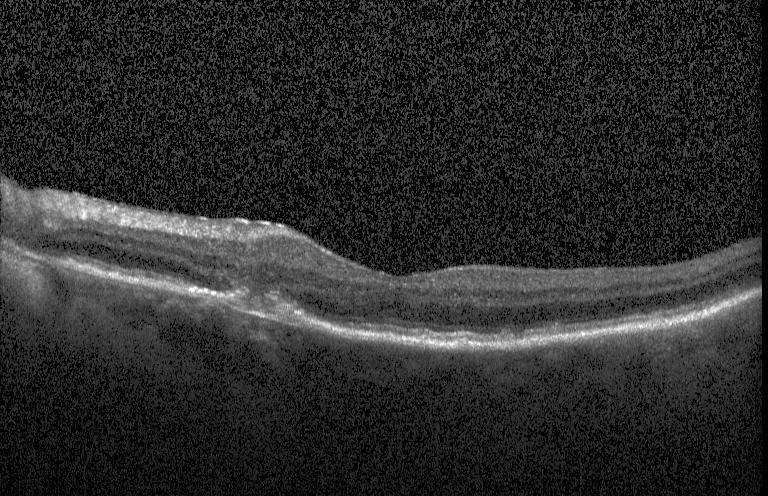

OCT finding: CNV.